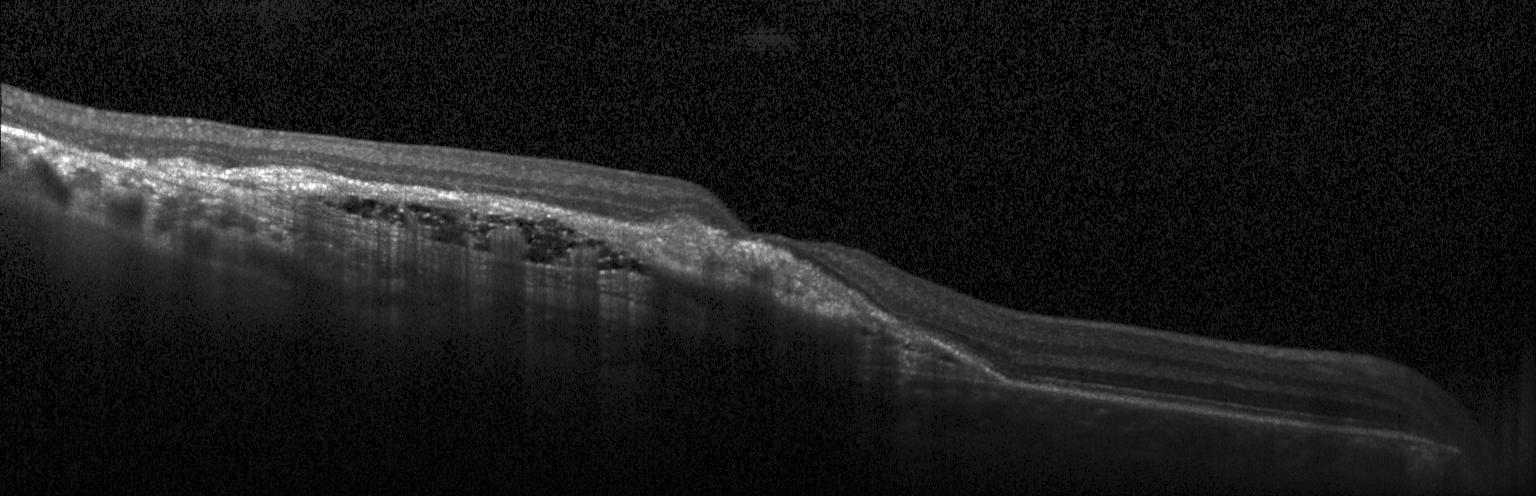 Finding: a choroidal neovascular membrane.